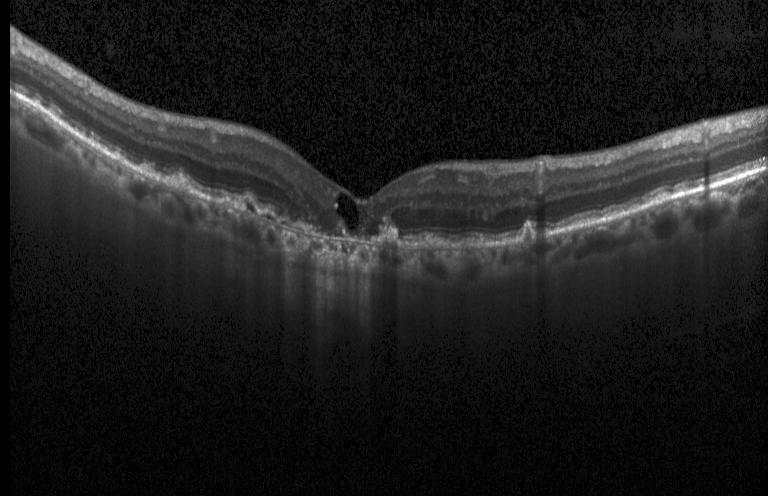
Retinal OCT cross-section · horizontal scan through the fovea · Heidelberg Spectralis · spectral-domain optical coherence tomography.
The scan shows CNV.